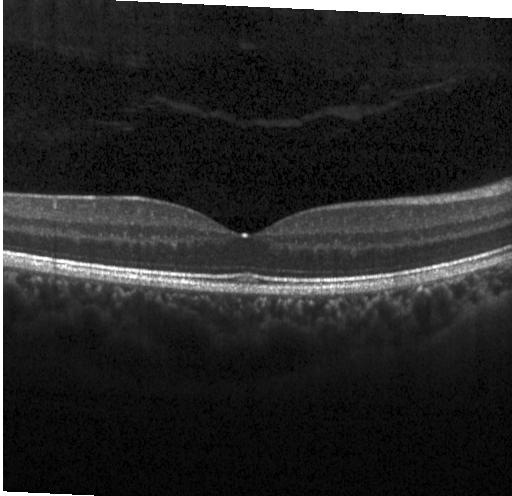
Retinal OCT cross-section; centered on the fovea. Dx: no evidence of CNV, DME, or drusen.